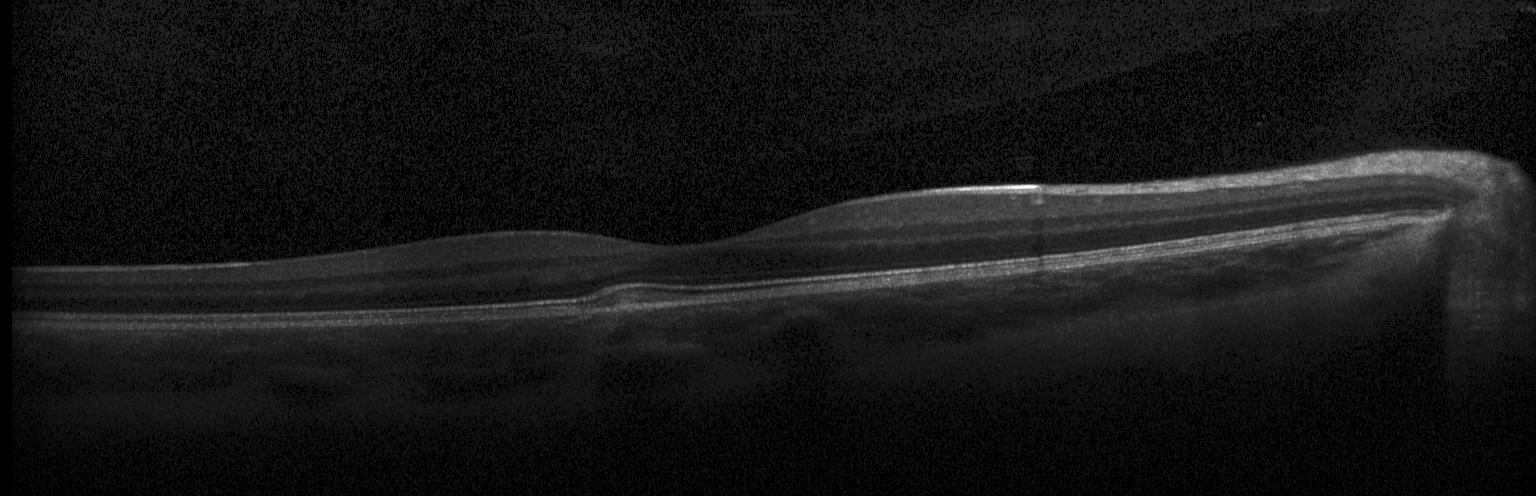
SD-OCT. Optical coherence tomography B-scan. Heidelberg Spectralis
Impression: no choroidal neovascularization, diabetic macular edema, or drusen.